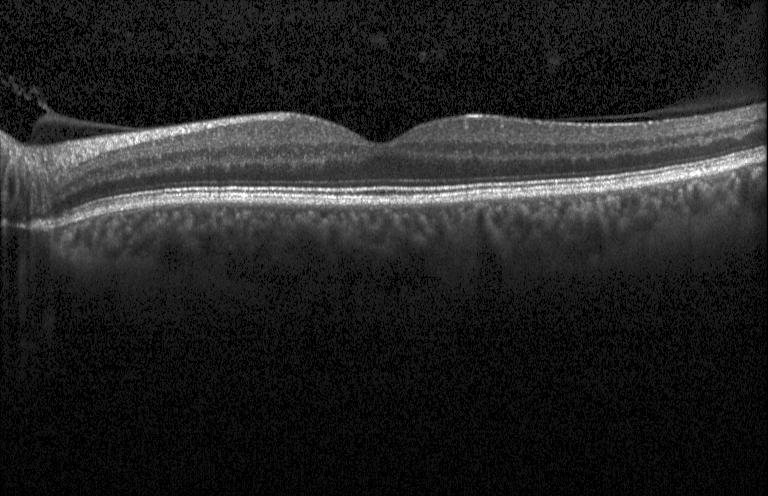 OCT line scan; acquired on a Heidelberg Spectralis; through the macula; SD-OCT.
Impression: neither CNV, DME, nor drusen.